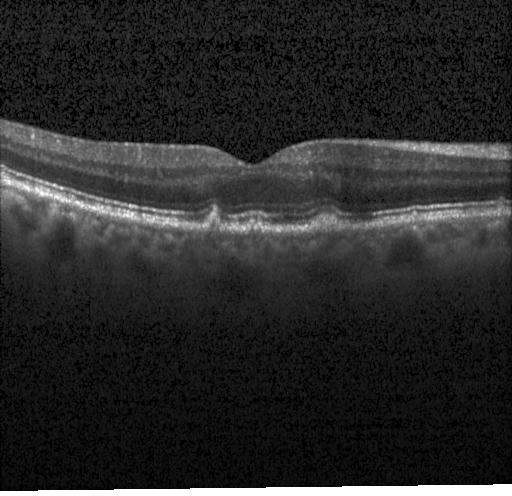
Optical coherence tomography B-scan. Assessment: drusen.